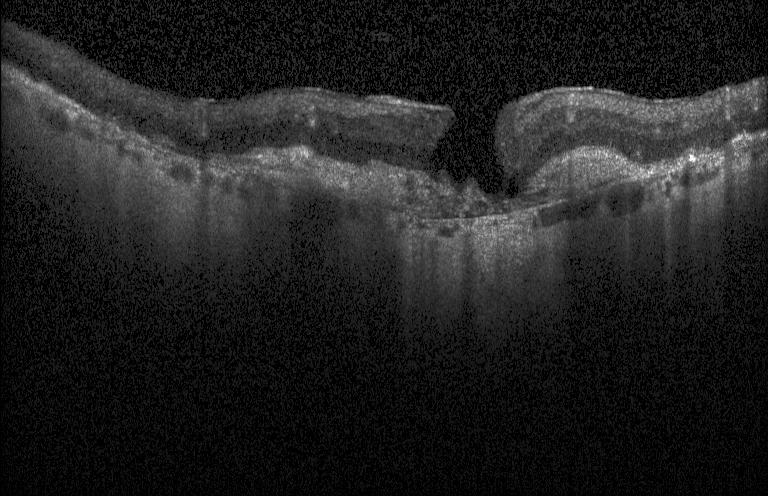 Spectral-domain optical coherence tomography. OCT B-scan. Fovea-centered. Heidelberg Spectralis
This B-scan demonstrates choroidal neovascularization (CNV).